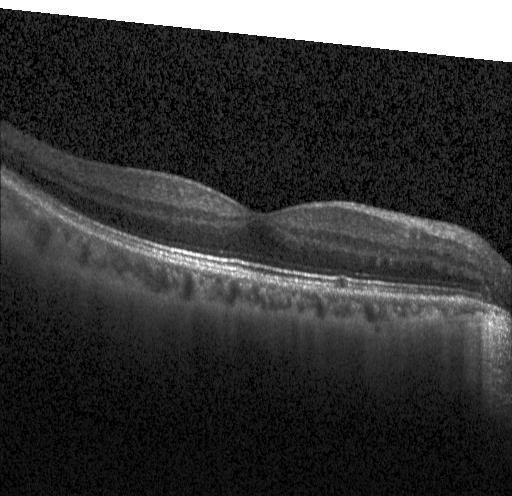 Optical coherence tomography scan. Instrument: Heidelberg Spectralis.
Diagnosis: no choroidal neovascularization, no diabetic macular edema, and no drusen.